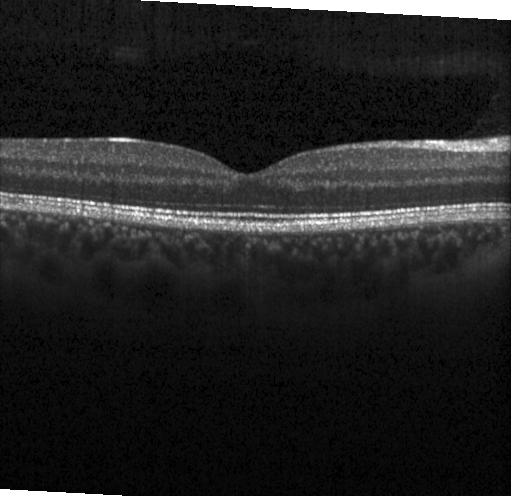 Spectral-domain optical coherence tomography, retinal OCT B-scan. Neither choroidal neovascularization, diabetic macular edema, nor drusen.